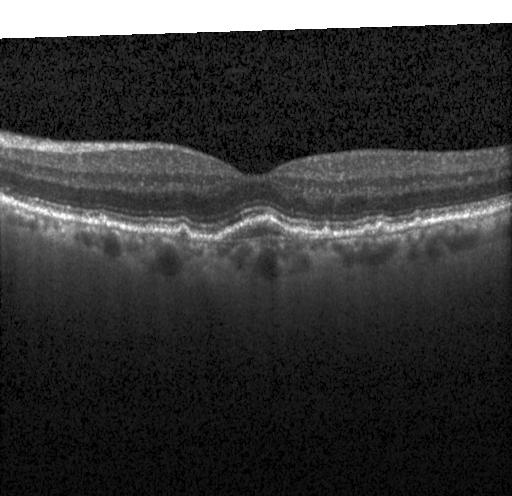 Finding: a choroidal neovascular membrane.